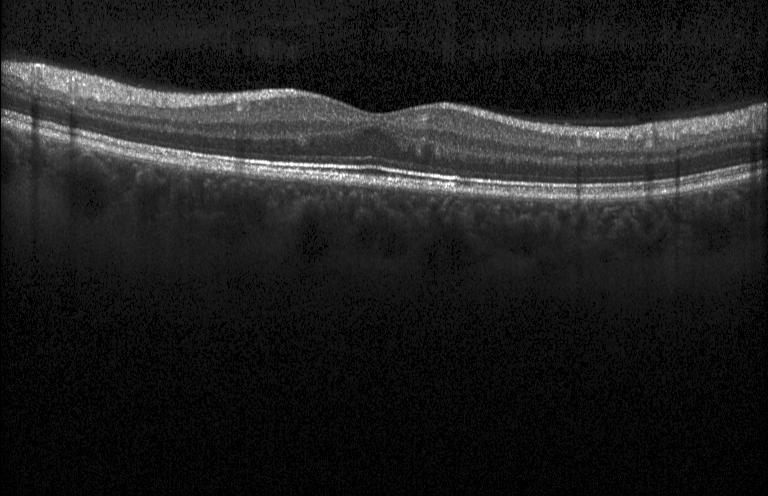 OCT B-scan — Impression: no evidence of choroidal neovascularization, diabetic macular edema, or drusen.